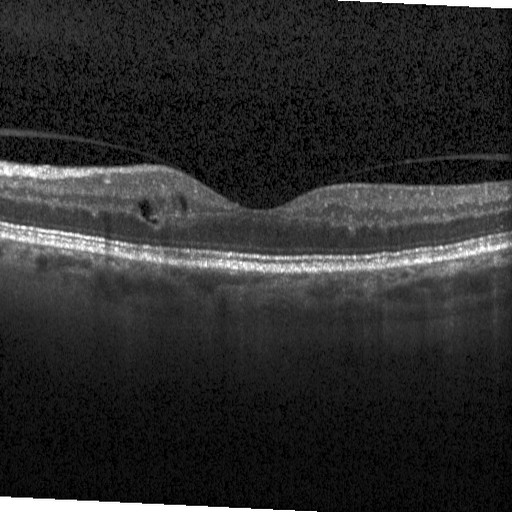

OCT B-scan · spectral-domain optical coherence tomography.
This B-scan demonstrates DME.